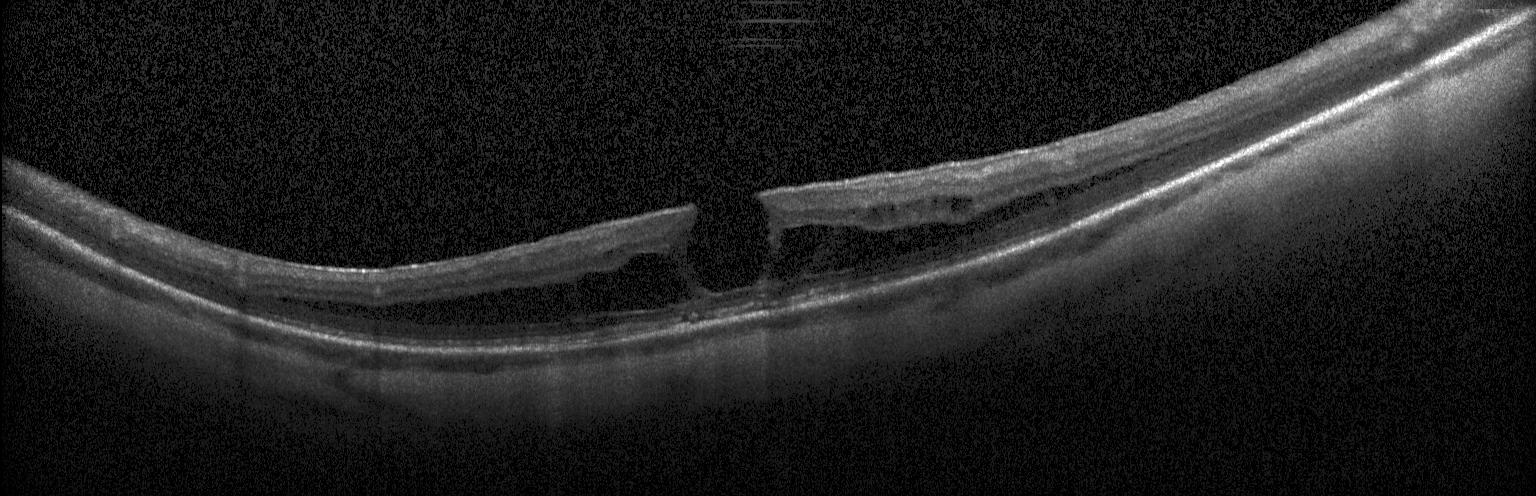
The scan shows DME.